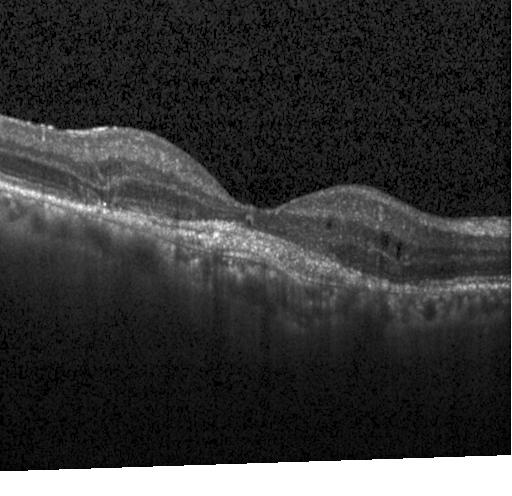

Acquired on a Heidelberg Spectralis; retinal OCT B-scan; fovea-centered; spectral-domain optical coherence tomography — Finding: CNV.